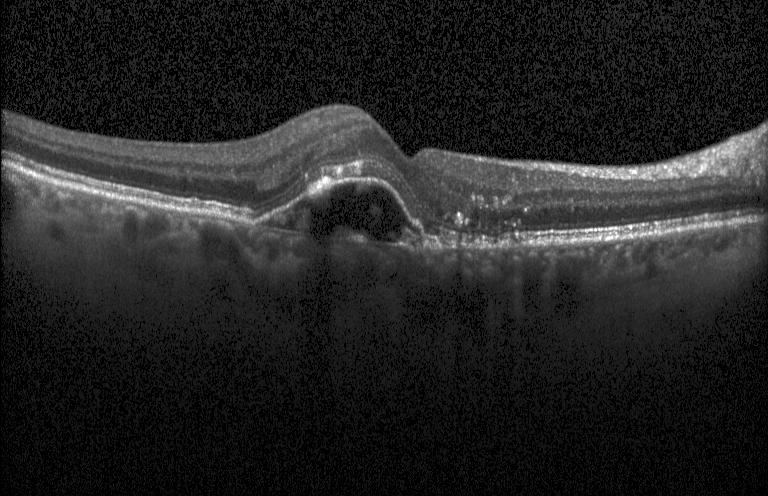 Optical coherence tomography B-scan. Acquired on a Heidelberg Spectralis. SD-OCT. Centered on the fovea.
Finding: choroidal neovascularization.